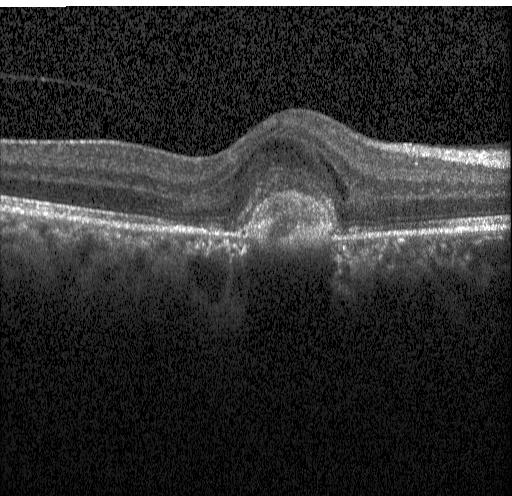 Macular scan. Optical coherence tomography B-scan. Instrument: Heidelberg Spectralis — CNV.